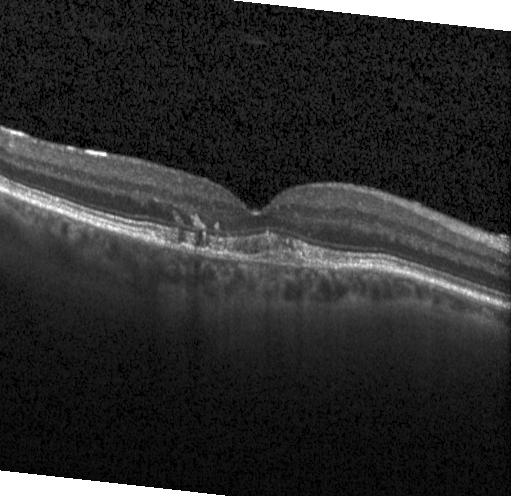
Retinal OCT cross-section
OCT finding: a choroidal neovascular membrane.